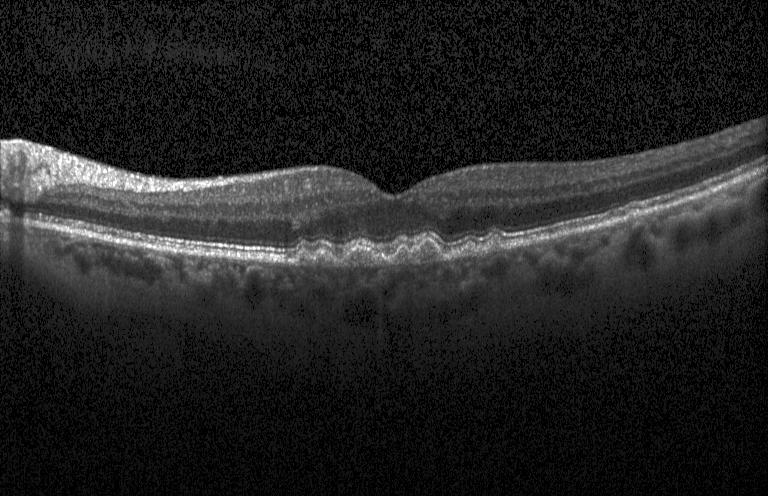 Multiple drusen.